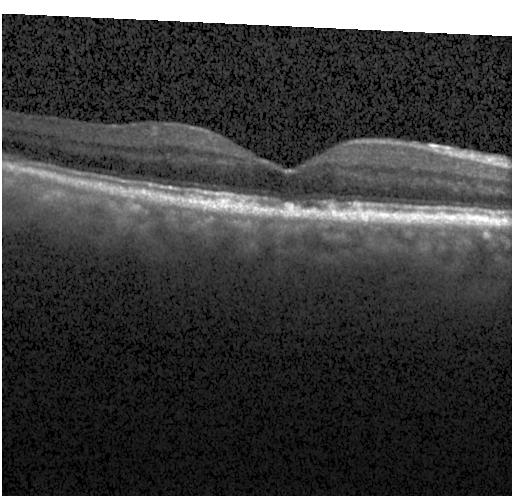

Fovea-centered. Heidelberg Spectralis. OCT B-scan. This B-scan demonstrates multiple drusen.